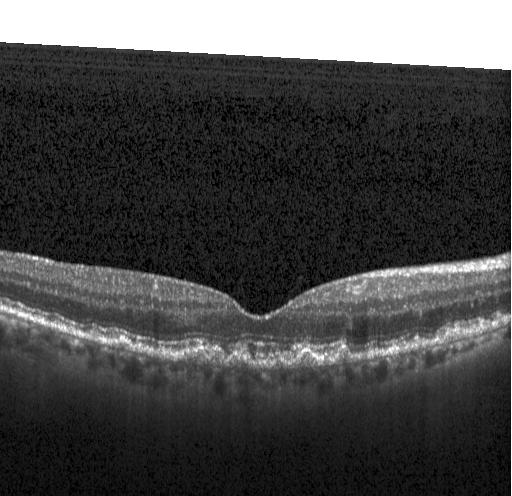
Dx: drusen.